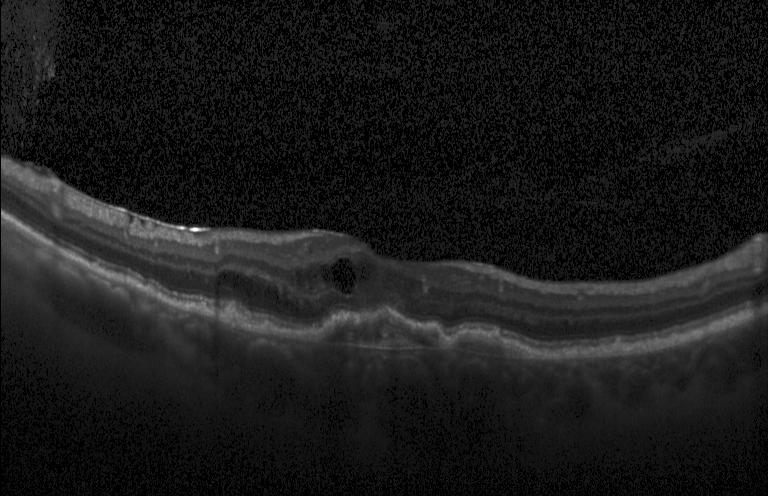 OCT finding: a choroidal neovascular membrane.